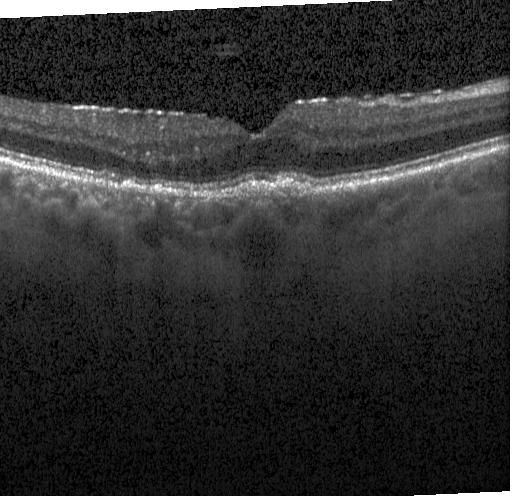
Dx: a choroidal neovascular membrane.